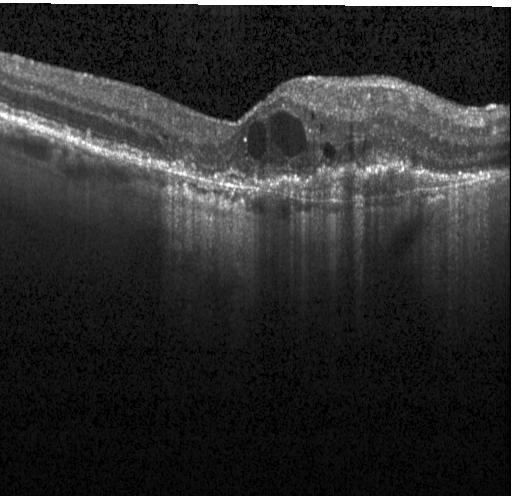 OCT finding: CNV.